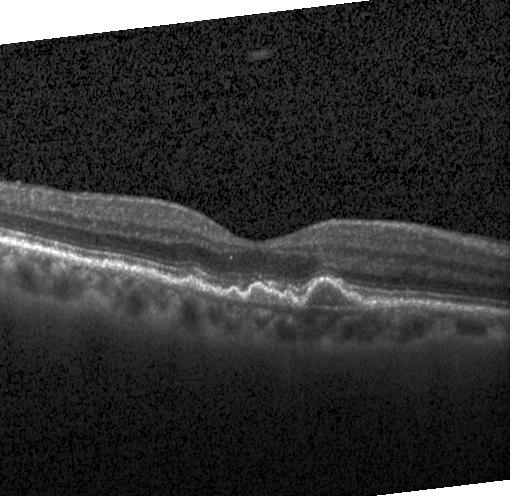

Diagnosis: sub-RPE drusenoid deposits.